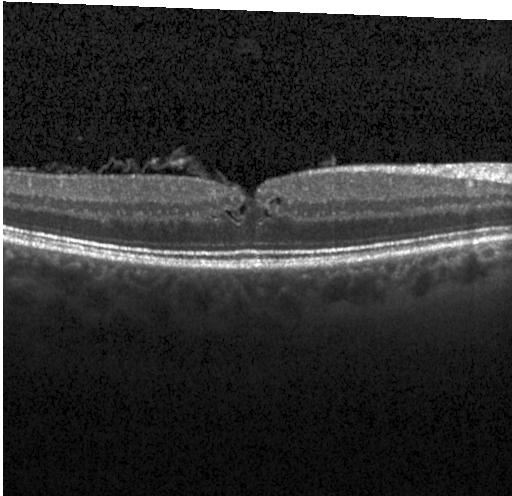

Heidelberg Spectralis; SD-OCT; through the macula; retinal OCT cross-section
Diagnosis: diabetic macular edema.